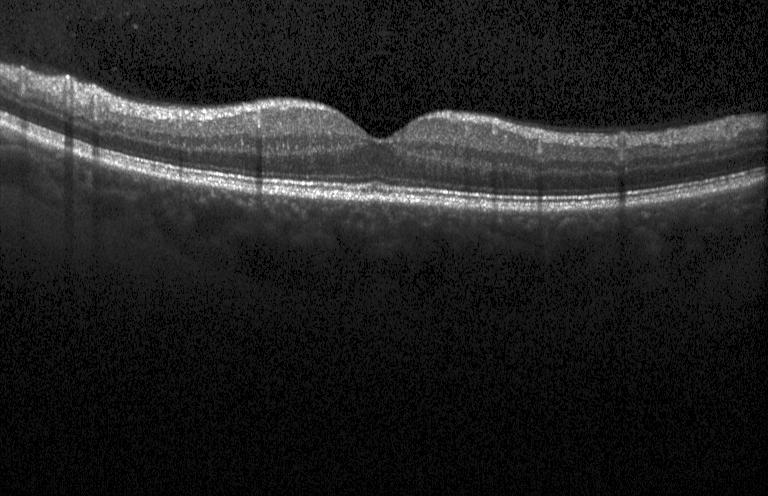 No evidence of CNV, DME, or drusen.